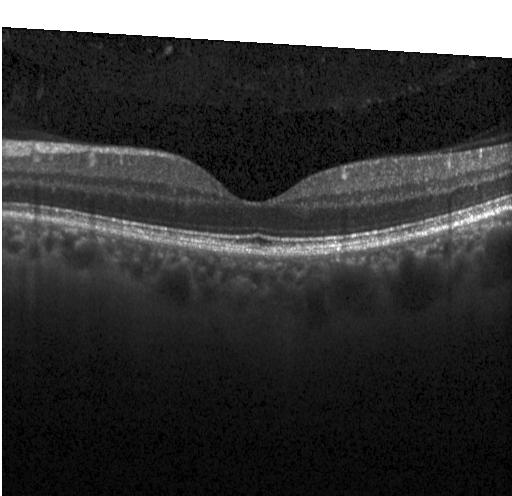
Optical coherence tomography scan; Heidelberg Spectralis.
OCT finding: no choroidal neovascularization, no diabetic macular edema, and no drusen.